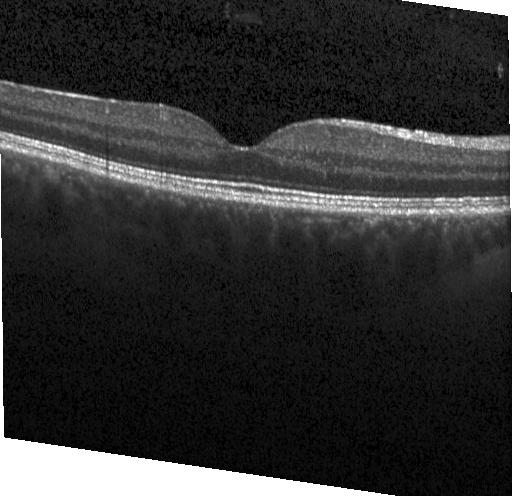 OCT B-scan, spectral-domain OCT, acquired on a Heidelberg Spectralis, centered on the fovea — The scan shows no CNV, DME, or drusen.